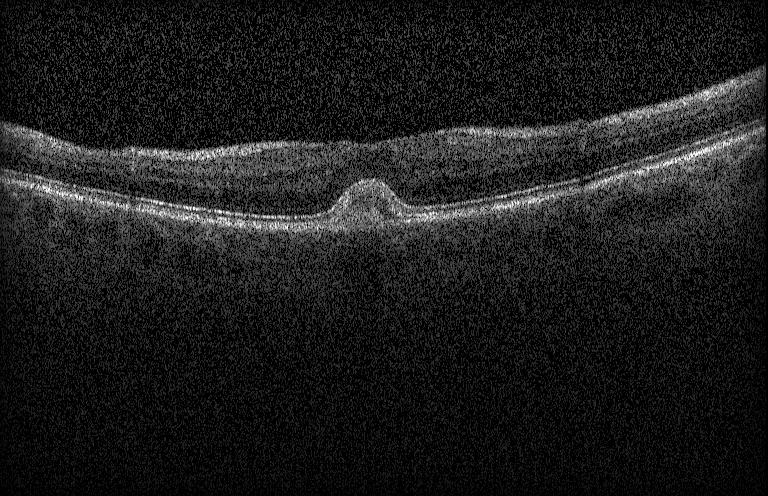 OCT B-scan · SD-OCT.
Finding: CNV.